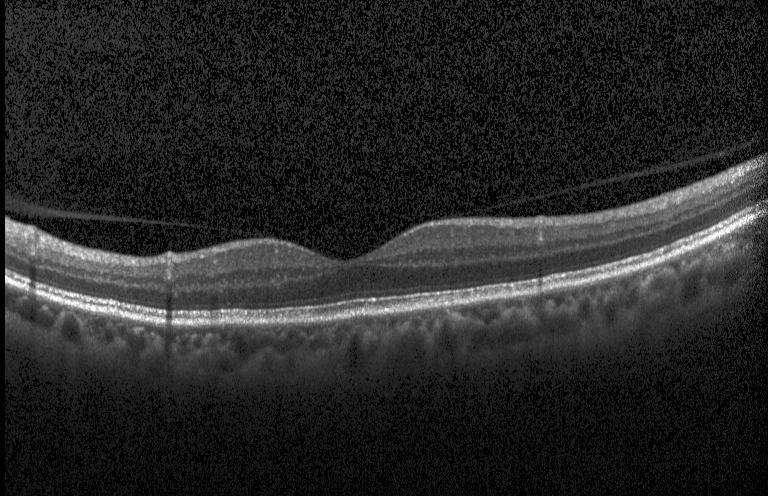

OCT line scan · acquired on a Heidelberg Spectralis. Diagnosis: neither choroidal neovascularization, diabetic macular edema, nor drusen.